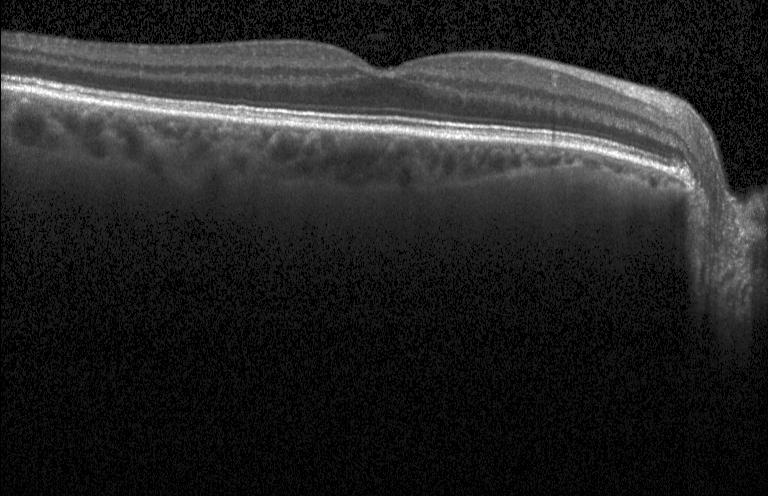

Dx: neither choroidal neovascularization, diabetic macular edema, nor drusen.